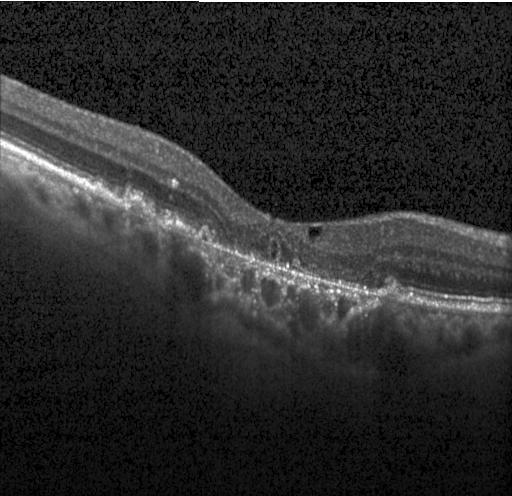

Spectral-domain OCT · OCT line scan. OCT finding: choroidal neovascularization (CNV).